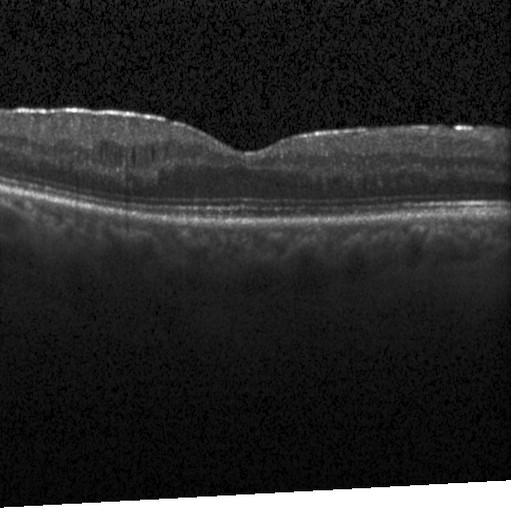 Through the macula. Heidelberg Spectralis OCT system. SD-OCT. Retinal OCT B-scan. Diagnosis: DME.